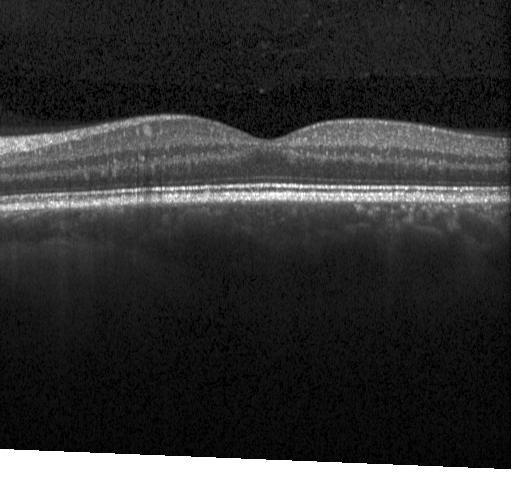

Optical coherence tomography B-scan
Macular OCT: no evidence of choroidal neovascularization, diabetic macular edema, or drusen.